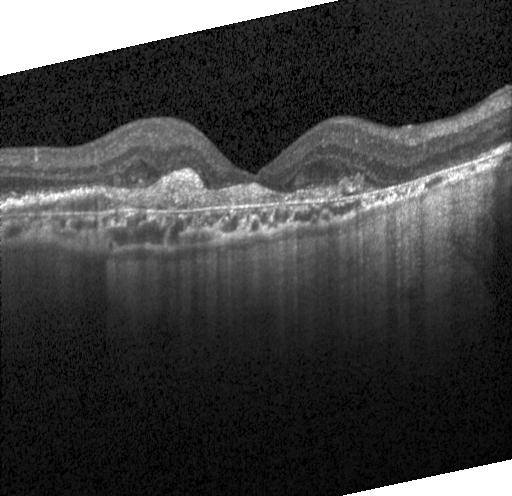

Impression: choroidal neovascularization (CNV).